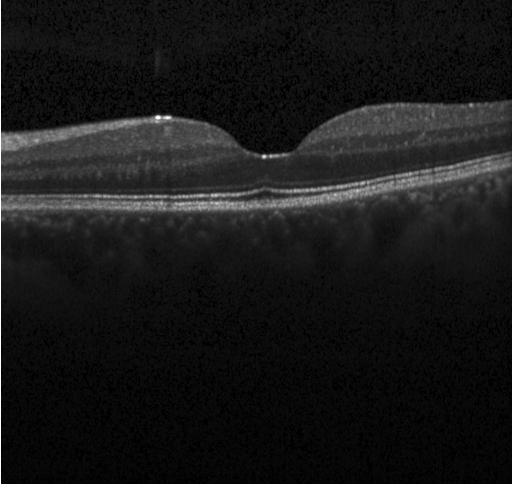
Heidelberg Spectralis, OCT B-scan, spectral-domain OCT.
Macular OCT: no choroidal neovascularization, no diabetic macular edema, and no drusen.